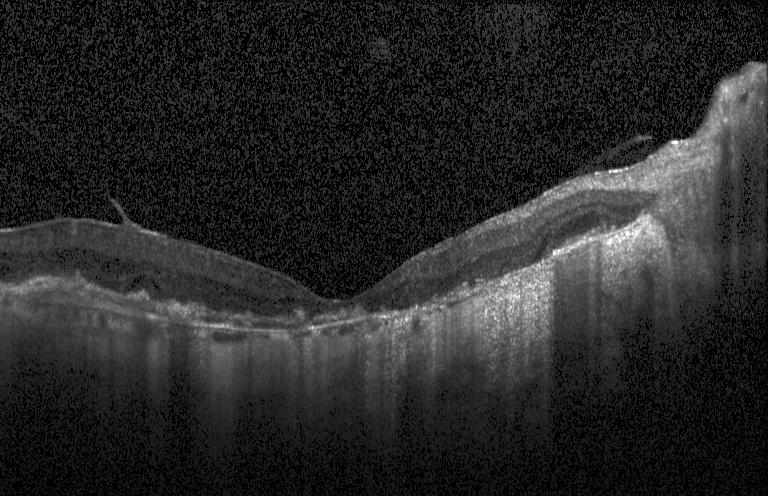
Retinal OCT cross-section. SD-OCT.
Macular OCT: a choroidal neovascular membrane.